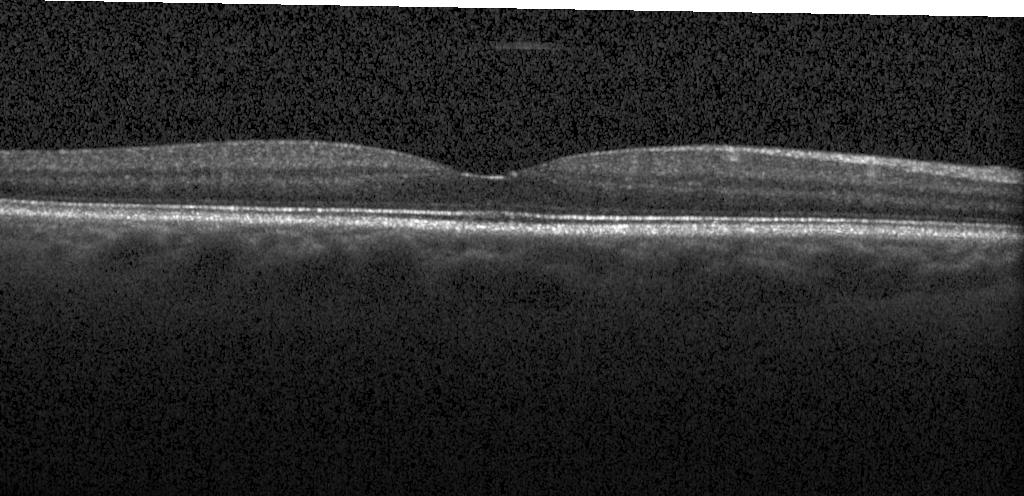
Optical coherence tomography B-scan, fovea-centered
Dx: no choroidal neovascularization, diabetic macular edema, or drusen.